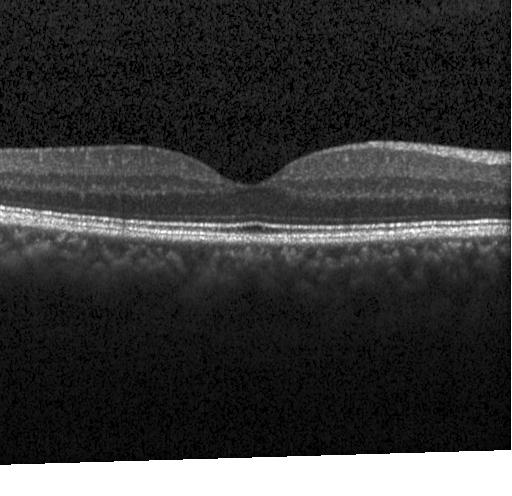
Spectral-domain OCT B-scan: no CNV, DME, or drusen.